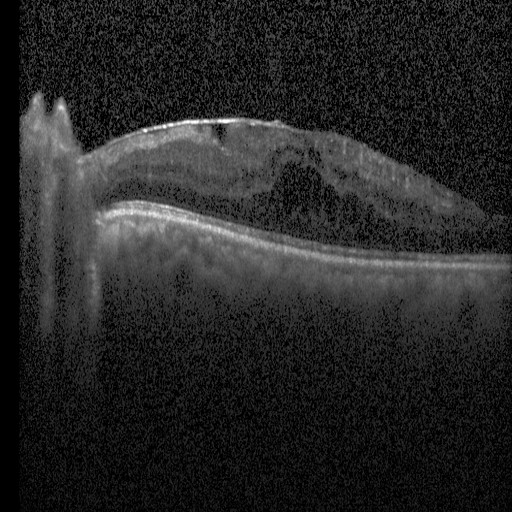

OCT B-scan, SD-OCT.
Impression: diabetic macular edema (DME).